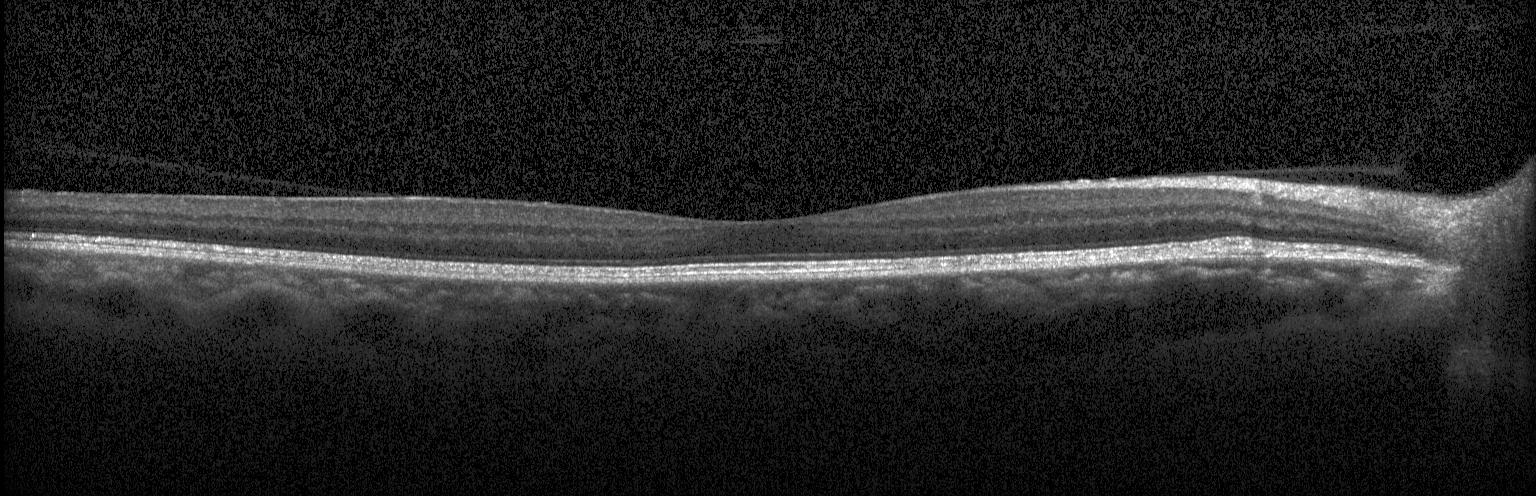 Retinal OCT B-scan. The scan shows no choroidal neovascularization, diabetic macular edema, or drusen.